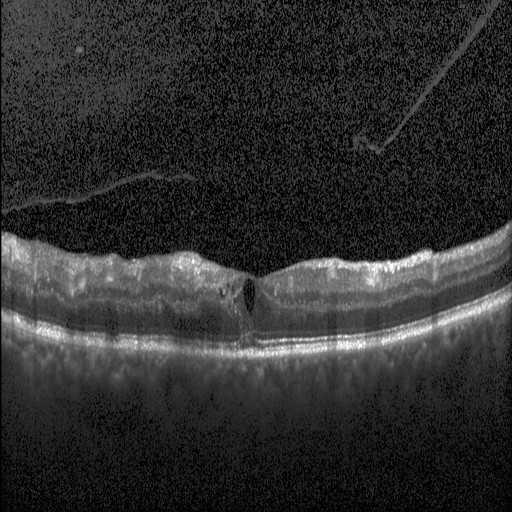
Diabetic macular edema (DME).